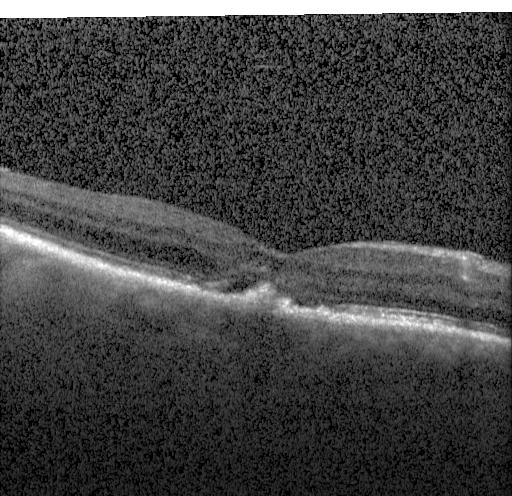

Impression: a choroidal neovascular membrane.